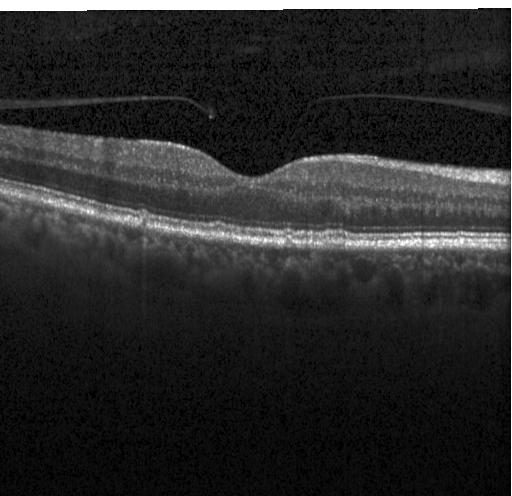 Macular OCT: multiple drusen.